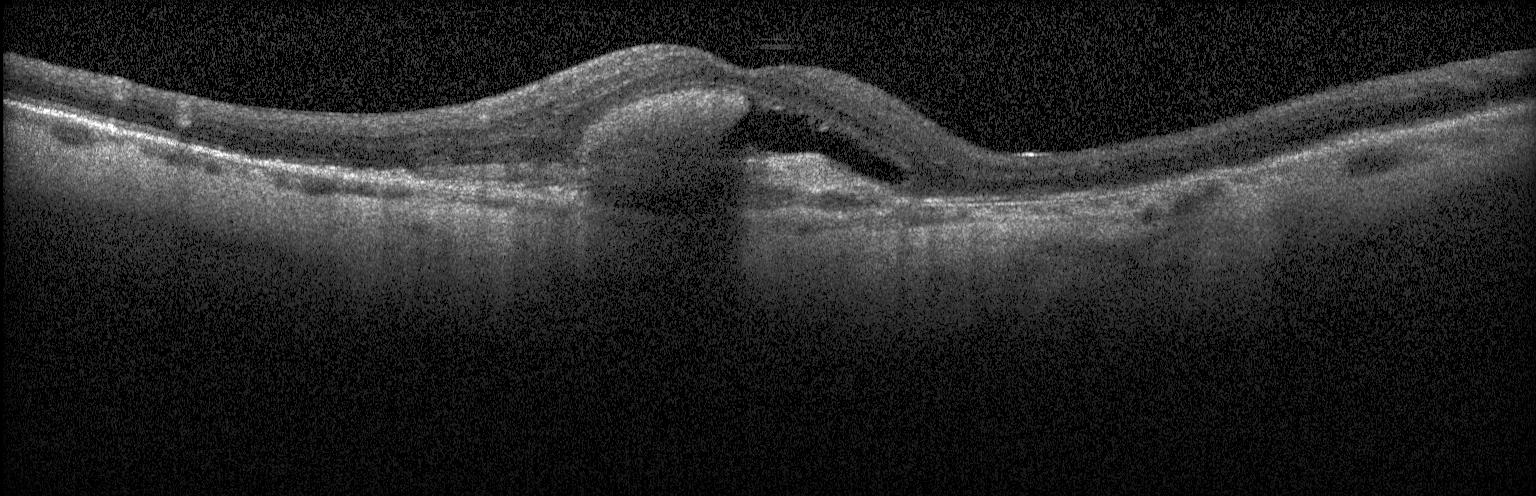
Fovea-centered, retinal OCT cross-section.
Finding: choroidal neovascularization (CNV).